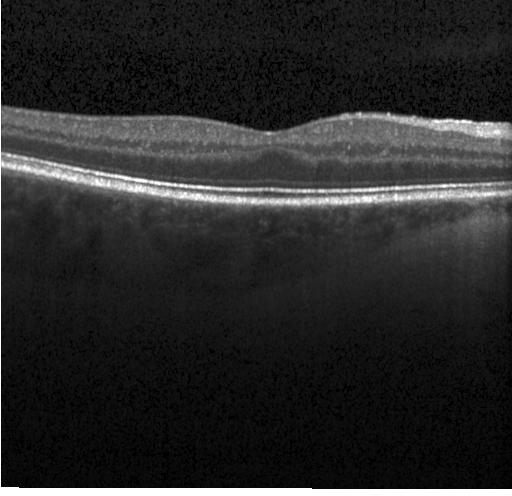

Diagnosis: no CNV, no DME, and no drusen.